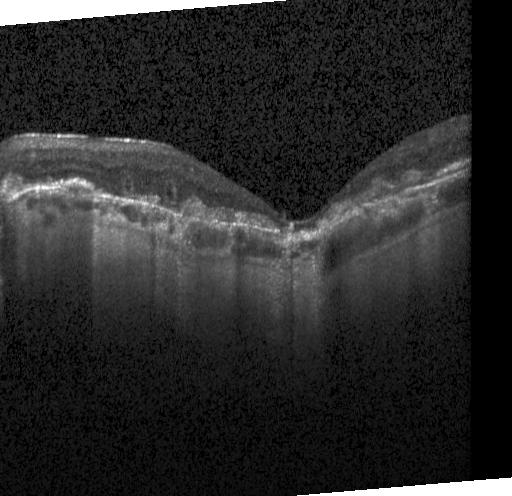
OCT B-scan. Finding: a choroidal neovascular membrane.